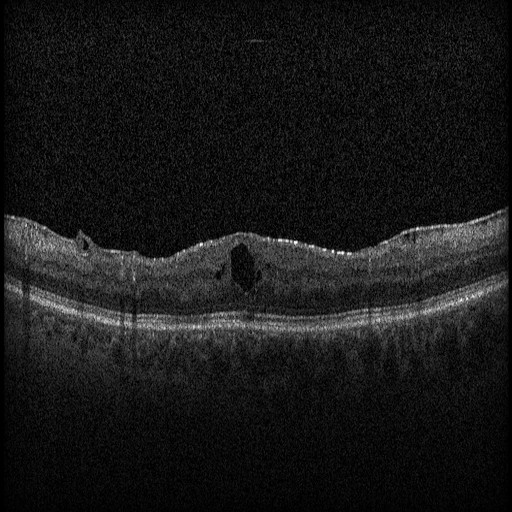 OCT B-scan. Heidelberg Spectralis. SD-OCT. Fovea-centered. Diagnosis: diabetic macular edema (DME).